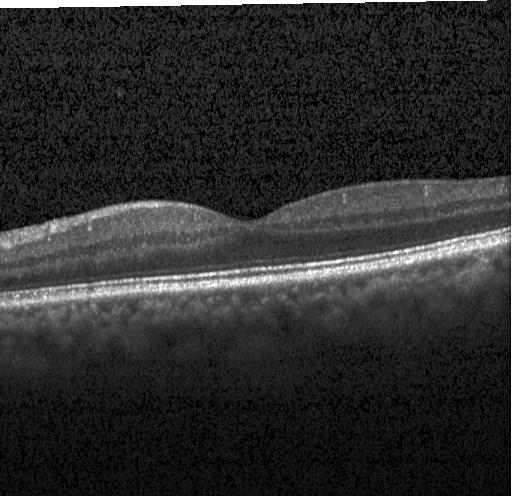
Macular OCT: no evidence of choroidal neovascularization, diabetic macular edema, or drusen.